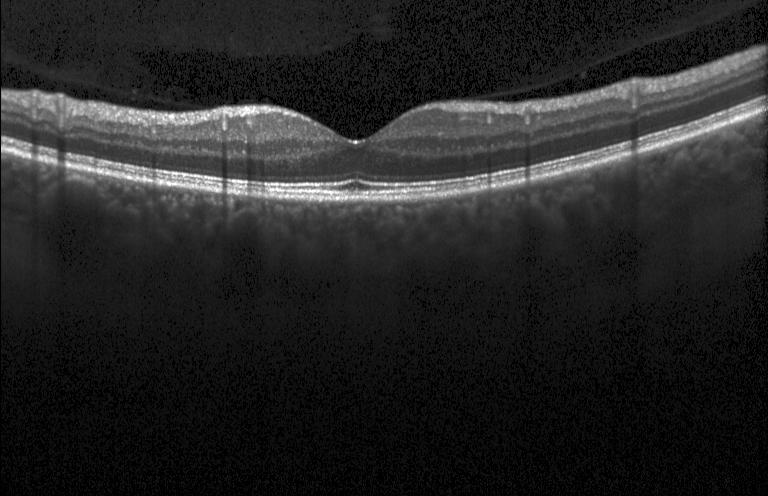 Spectral-domain OCT. Optical coherence tomography B-scan. Heidelberg Spectralis. Macular scan. Finding: no choroidal neovascularization, no diabetic macular edema, and no drusen.